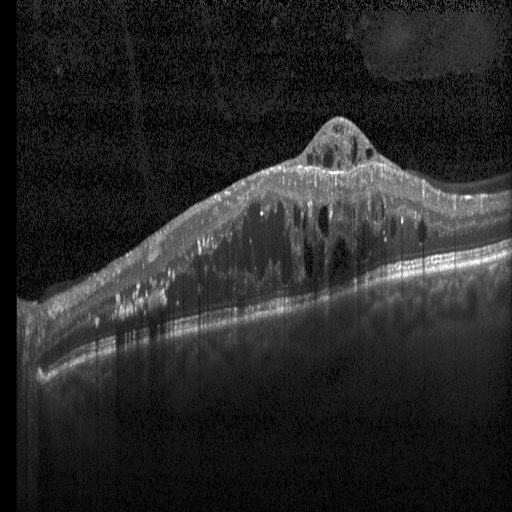 Assessment: diabetic macular edema (DME).